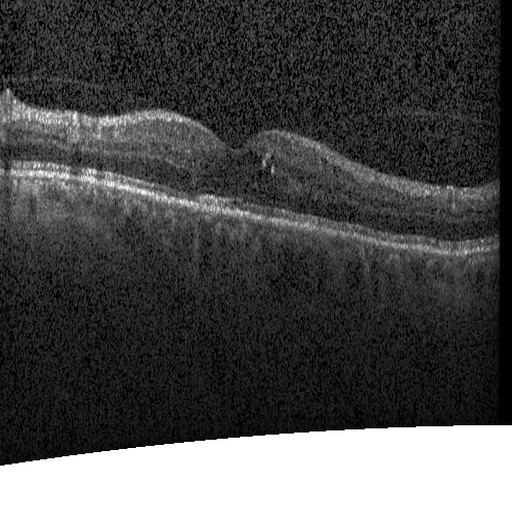

OCT B-scan, macular scan. The scan shows diabetic macular edema.